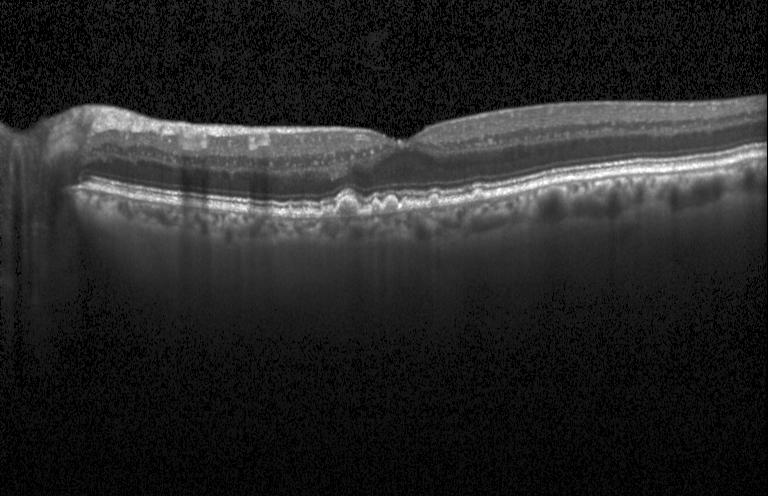

Assessment: multiple drusen.